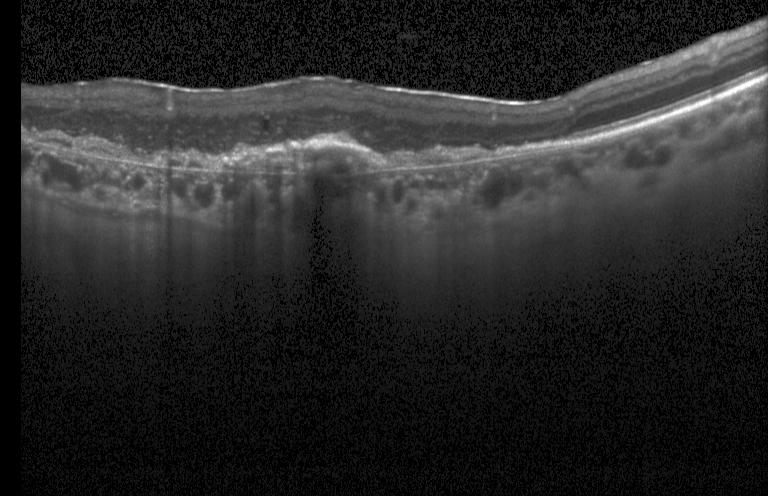

OCT line scan, acquired on a Heidelberg Spectralis, SD-OCT, fovea-centered
A choroidal neovascular membrane.